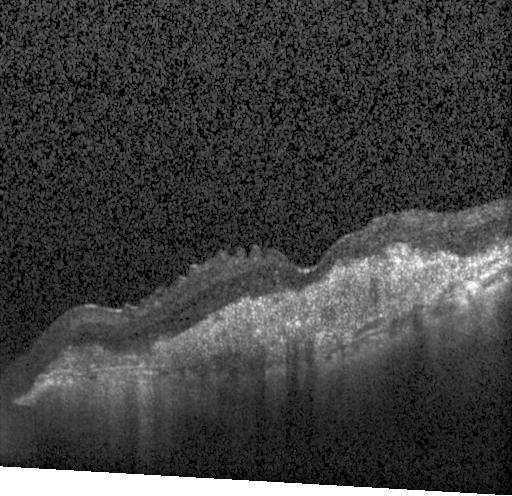
Optical coherence tomography B-scan · instrument: Heidelberg Spectralis. Macular OCT: a choroidal neovascular membrane.